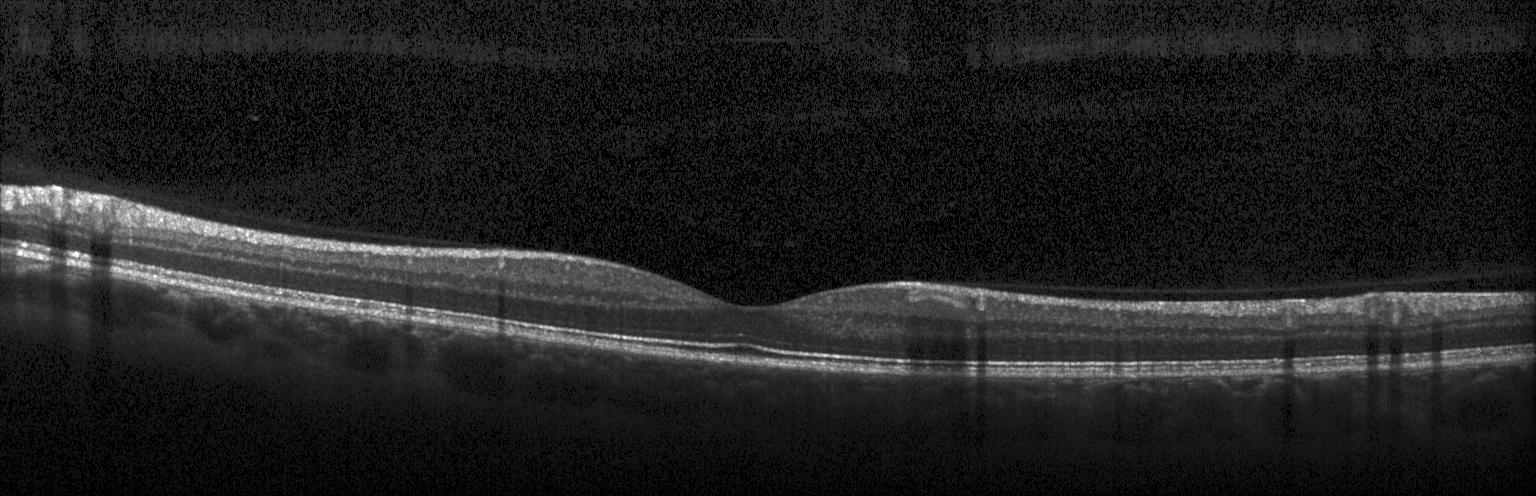

Optical coherence tomography scan; spectral-domain optical coherence tomography; centered on the fovea — Assessment: no choroidal neovascularization, no diabetic macular edema, and no drusen.